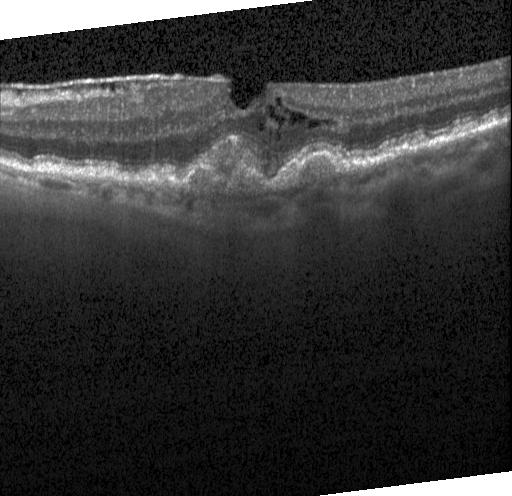
Macular scan. Optical coherence tomography B-scan
The scan shows a choroidal neovascular membrane.